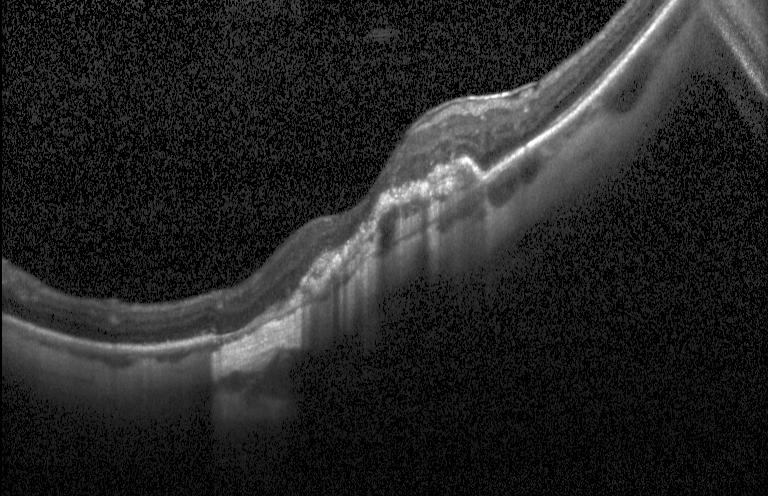
This B-scan demonstrates a choroidal neovascular membrane.